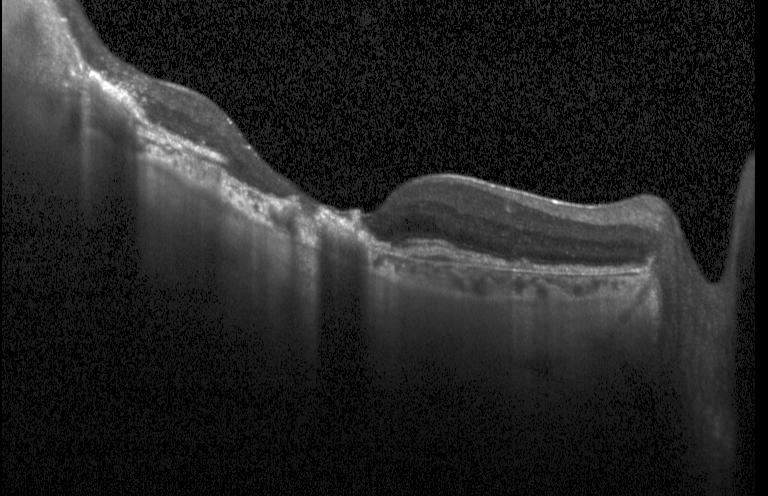

Macular OCT demonstrating a choroidal neovascular membrane.